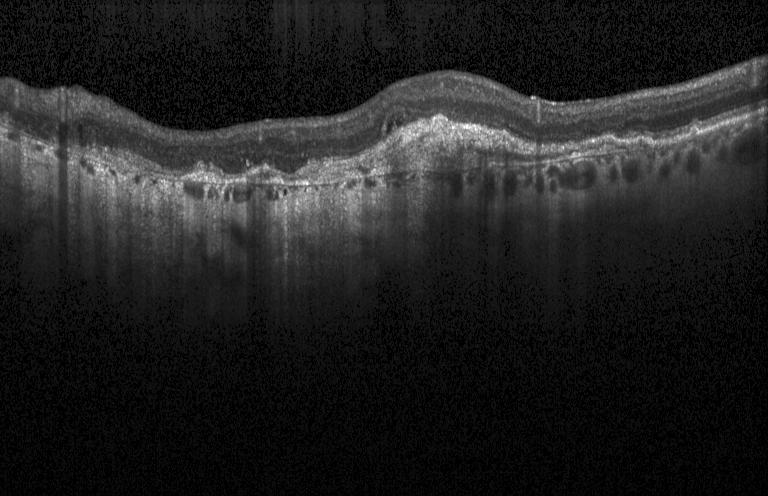 Instrument: Heidelberg Spectralis. OCT line scan. Assessment: choroidal neovascularization (CNV).